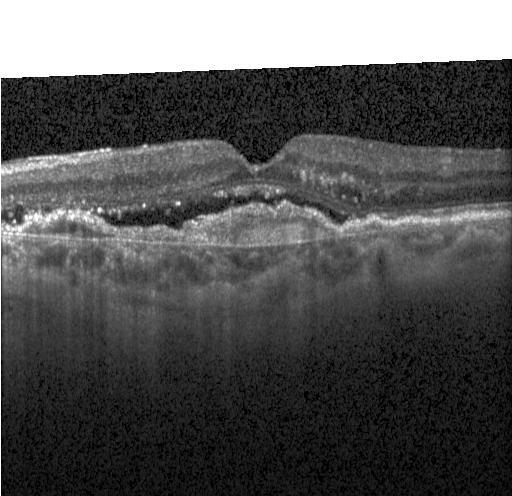 Optical coherence tomography B-scan.
Finding: choroidal neovascularization (CNV).